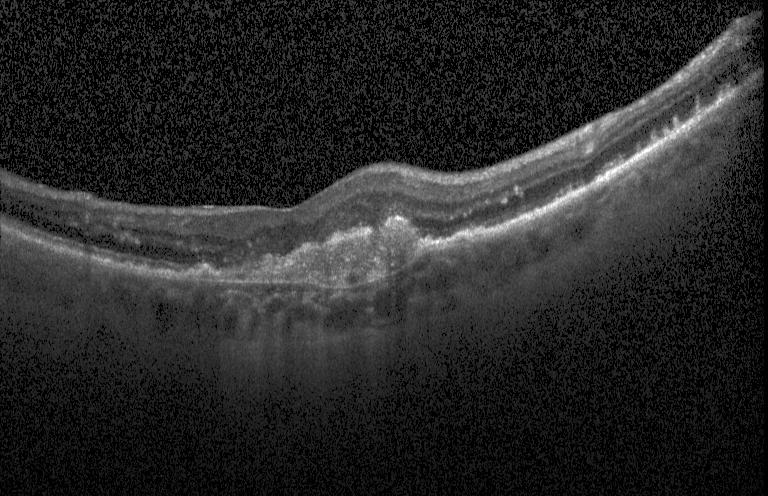

Acquired on a Heidelberg Spectralis · retinal OCT B-scan
This B-scan demonstrates choroidal neovascularization.